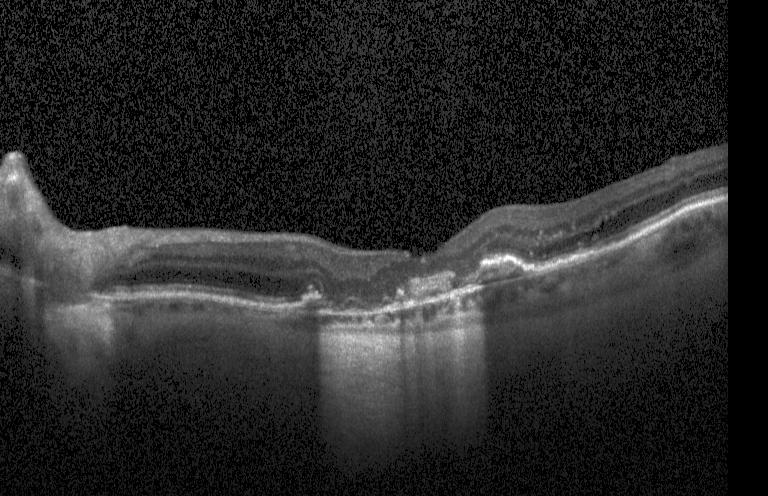
Choroidal neovascularization (CNV).